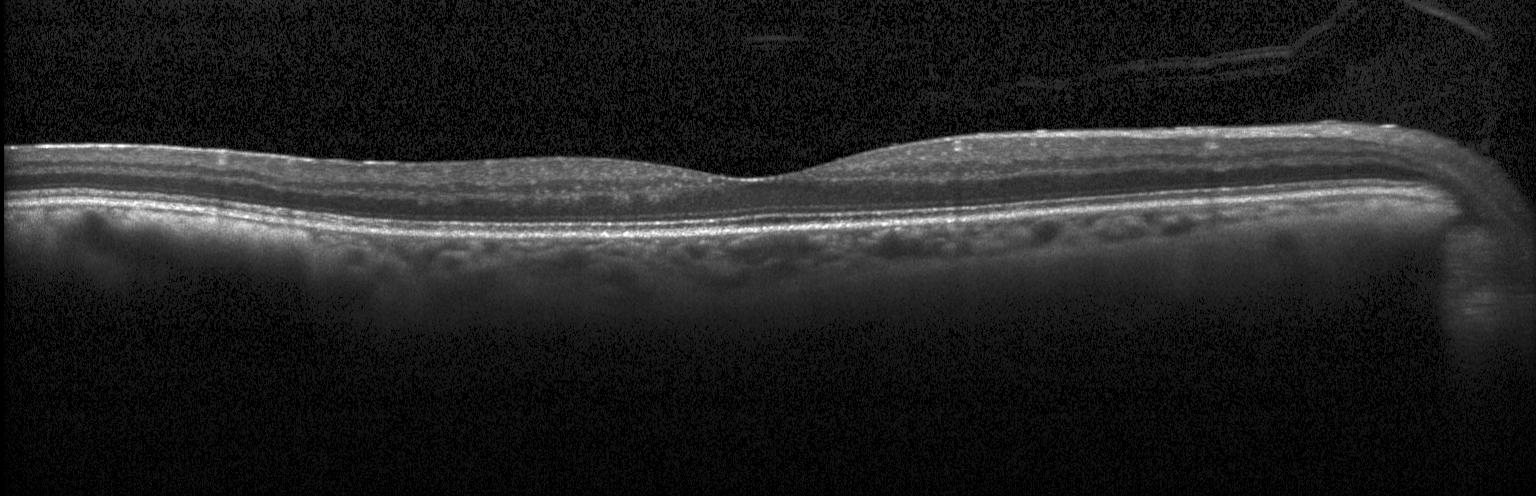 OCT line scan, acquired on a Heidelberg Spectralis. Dx: no choroidal neovascularization, no diabetic macular edema, and no drusen.